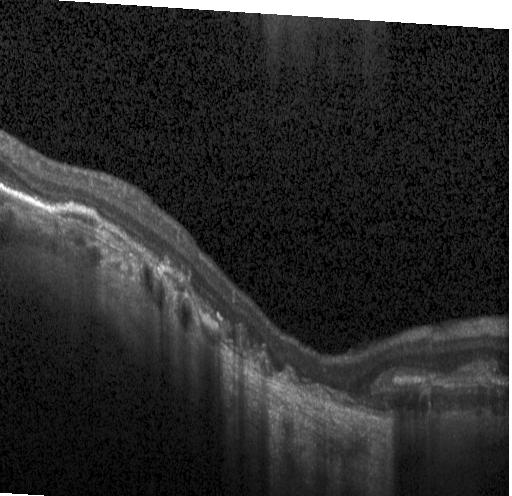

Centered on the fovea · OCT line scan · Heidelberg Spectralis OCT system · SD-OCT. The scan shows choroidal neovascularization (CNV).